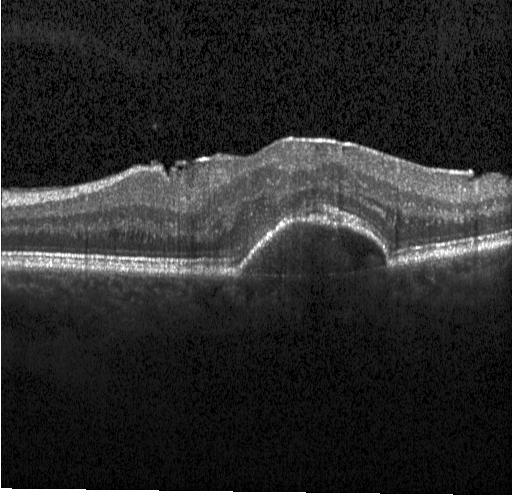 Acquired on a Heidelberg Spectralis · fovea-centered · SD-OCT · optical coherence tomography scan — Macular OCT: a choroidal neovascular membrane.